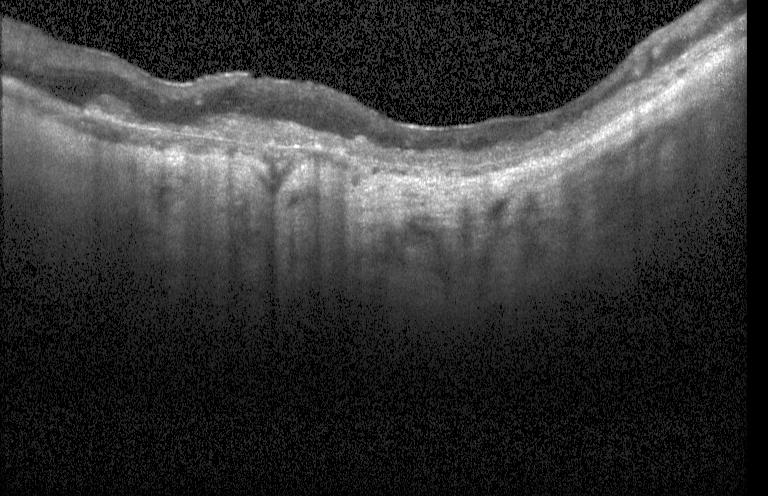 Through the macula · spectral-domain optical coherence tomography · retinal OCT B-scan — Finding: CNV.